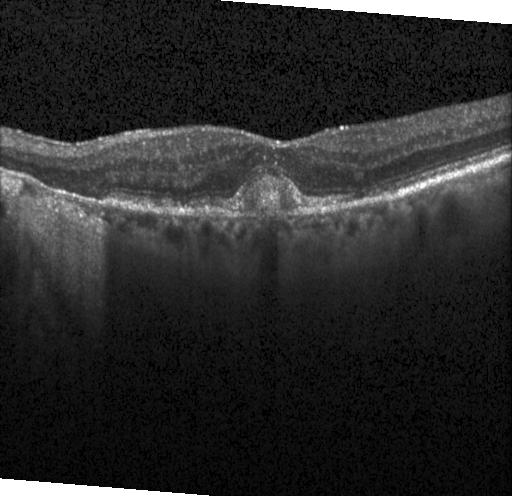
Optical coherence tomography scan
Assessment: choroidal neovascularization (CNV).